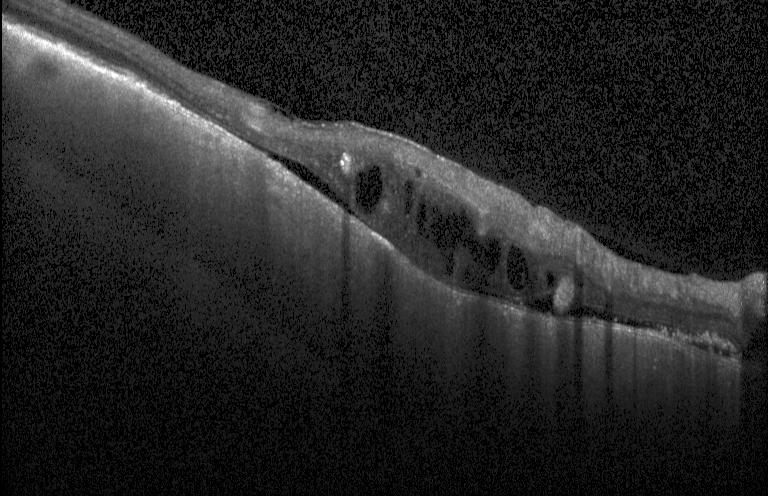
OCT B-scan — OCT finding: a choroidal neovascular membrane.